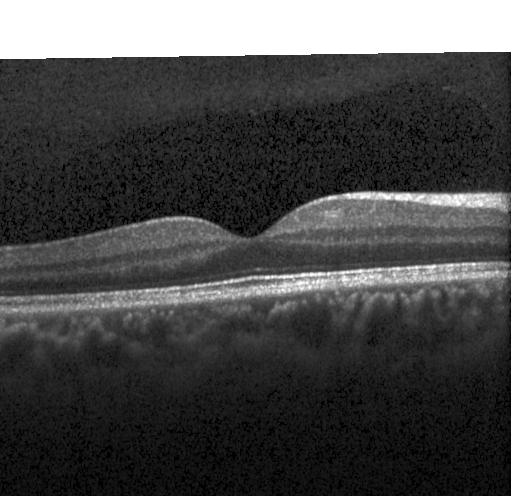 Dx: no choroidal neovascularization, diabetic macular edema, or drusen.